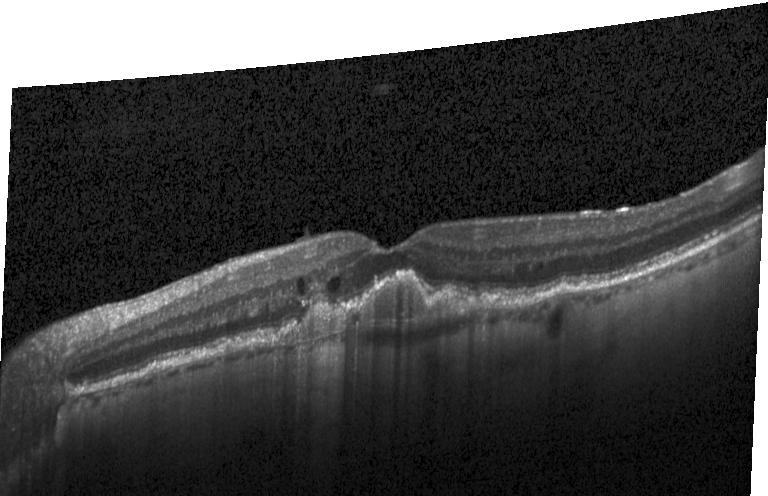
Optical coherence tomography B-scan; spectral-domain OCT; instrument: Heidelberg Spectralis — Assessment: CNV.